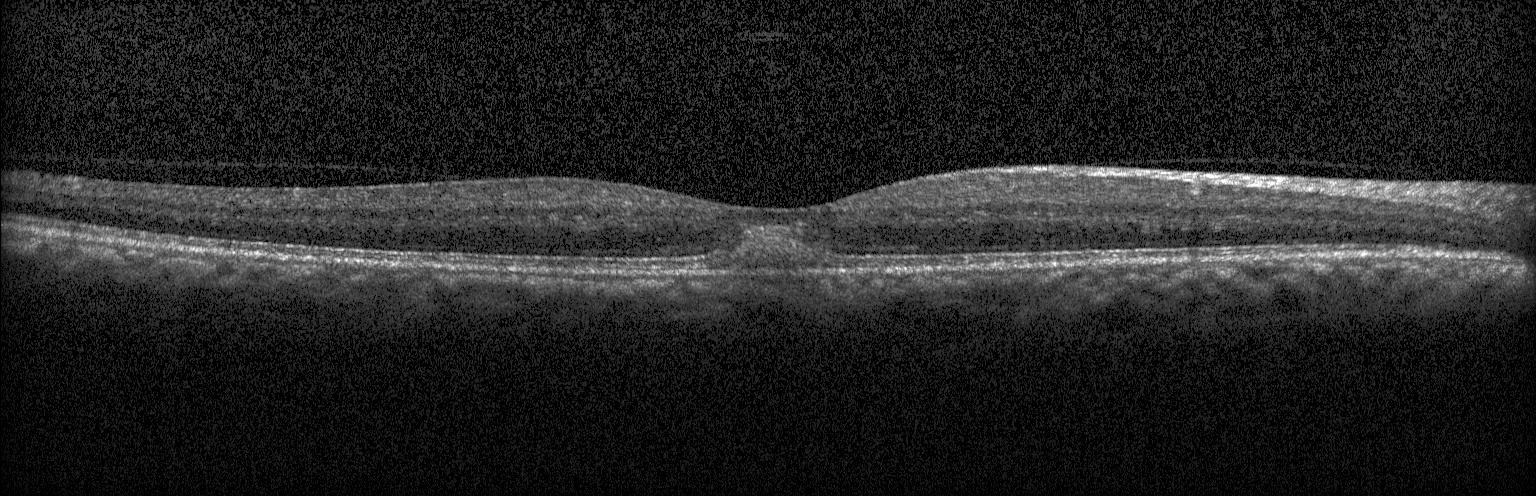

Fovea-centered, retinal OCT cross-section, Heidelberg Spectralis. Finding: a choroidal neovascular membrane.